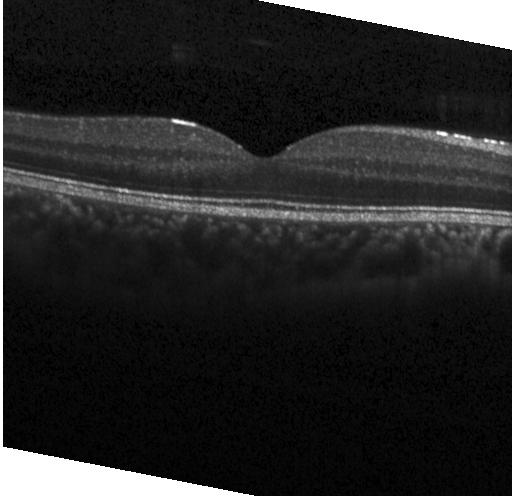 No evidence of CNV, DME, or drusen.